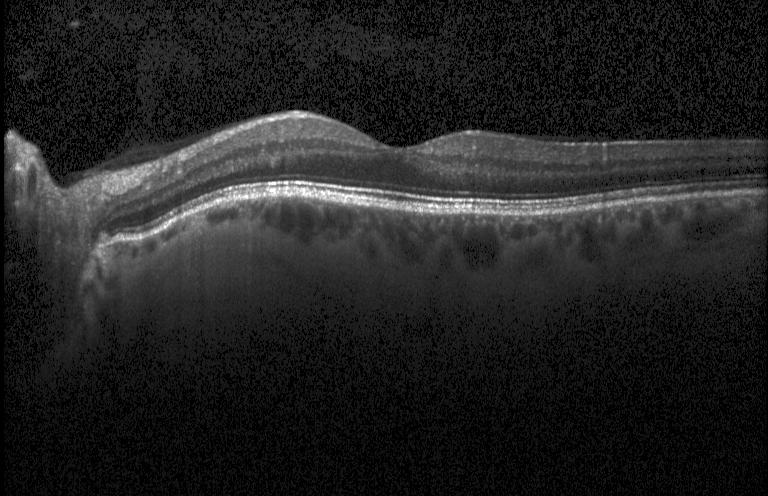

OCT B-scan — Finding: no choroidal neovascularization, no diabetic macular edema, and no drusen.